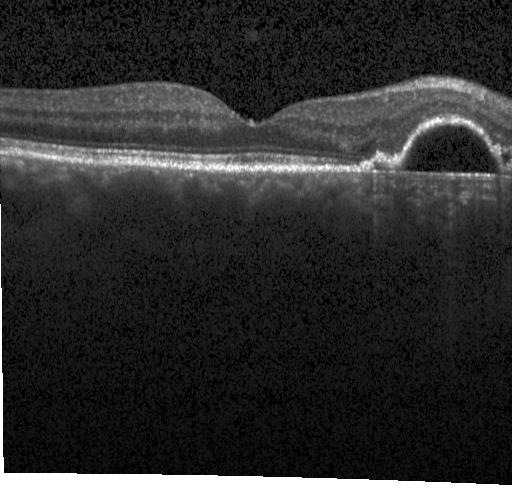

Macular OCT: a choroidal neovascular membrane.